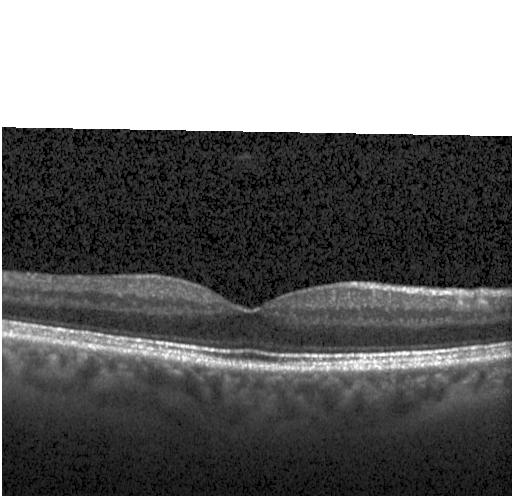
Neither choroidal neovascularization, diabetic macular edema, nor drusen.